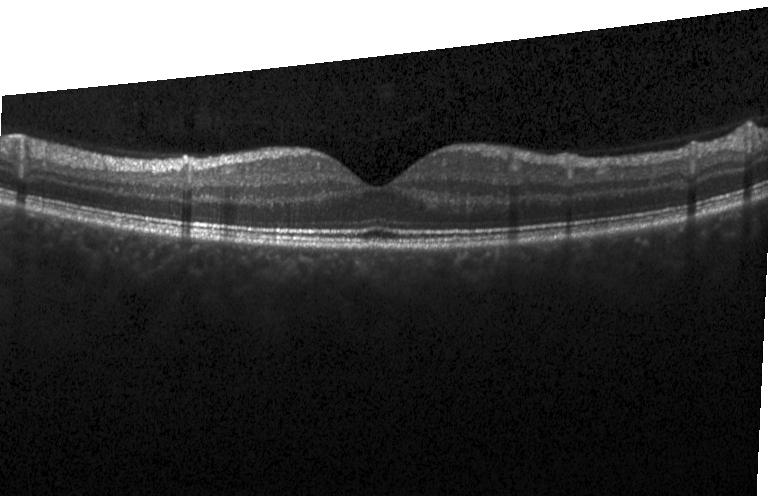

Dx: no evidence of CNV, DME, or drusen.